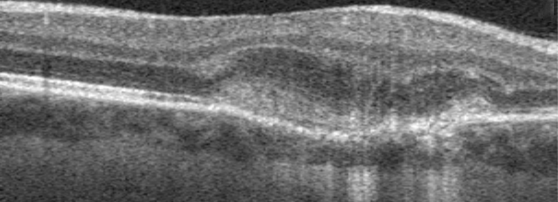 Retinal OCT B-scan — Finding: AMD.